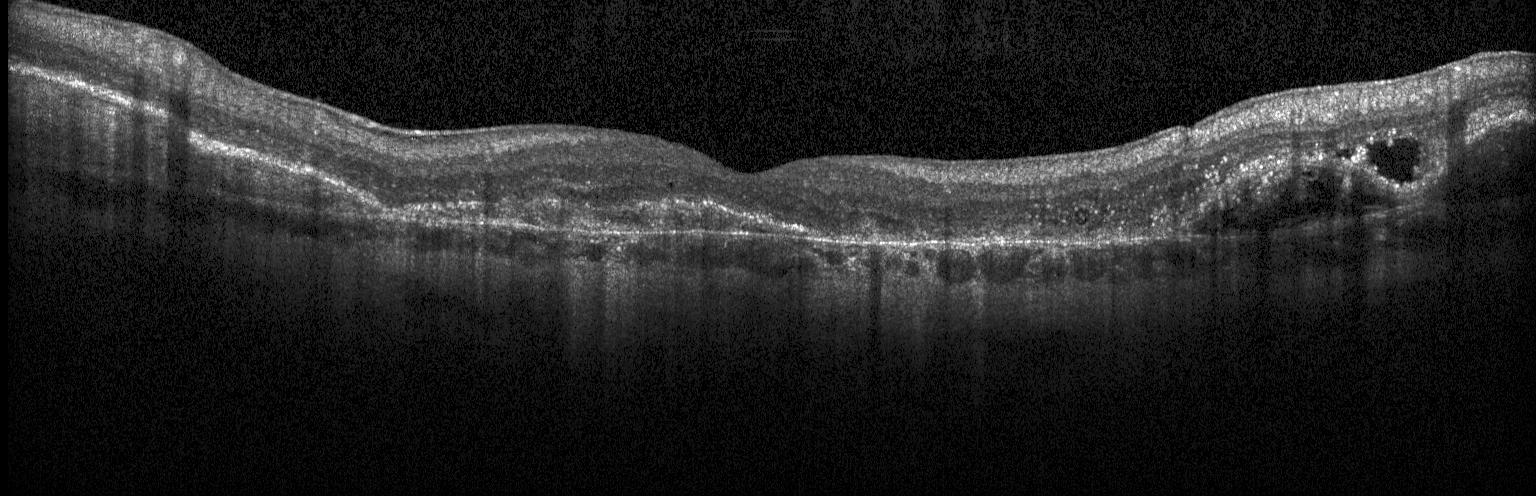

Optical coherence tomography B-scan. Spectral-domain optical coherence tomography. Horizontal scan through the fovea
Diagnosis: CNV.